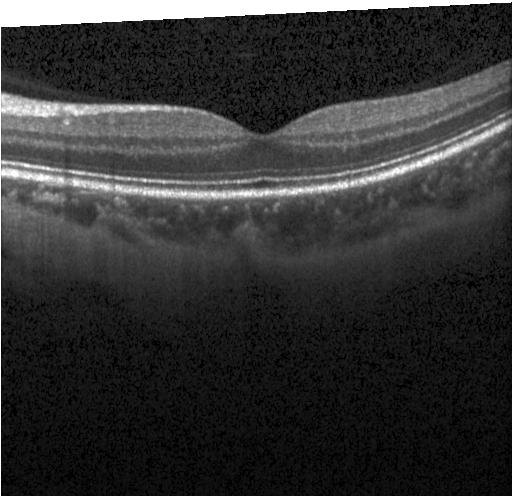
Spectral-domain OCT · retinal OCT cross-section · fovea-centered · instrument: Heidelberg Spectralis.
Impression: no CNV, no DME, and no drusen.